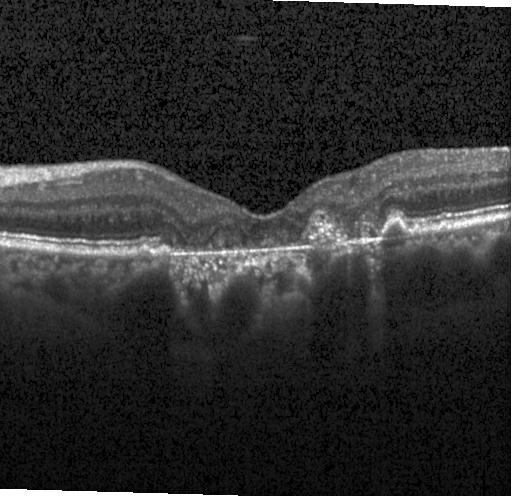
Optical coherence tomography B-scan, centered on the fovea
Assessment: choroidal neovascularization (CNV).